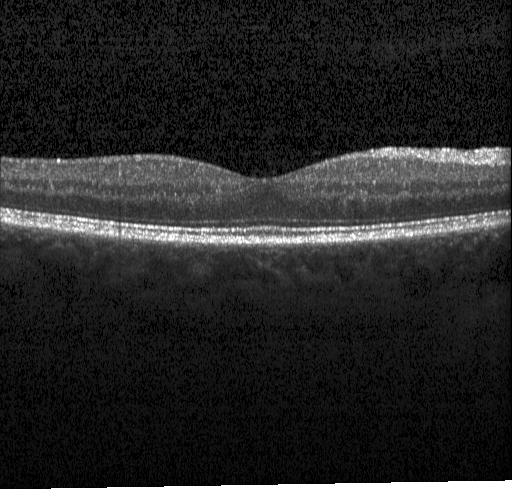
Retinal OCT cross-section showing no evidence of CNV, DME, or drusen.